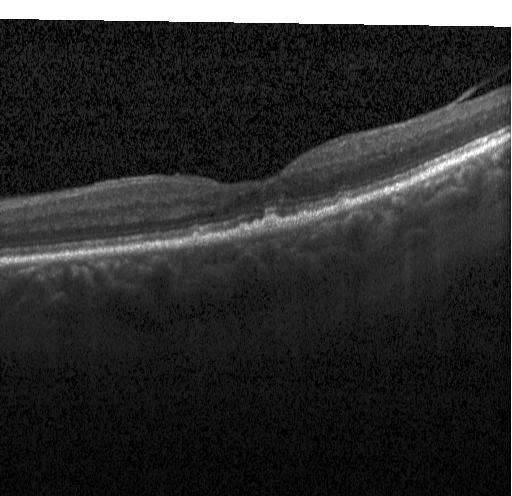

OCT B-scan showing multiple drusen.